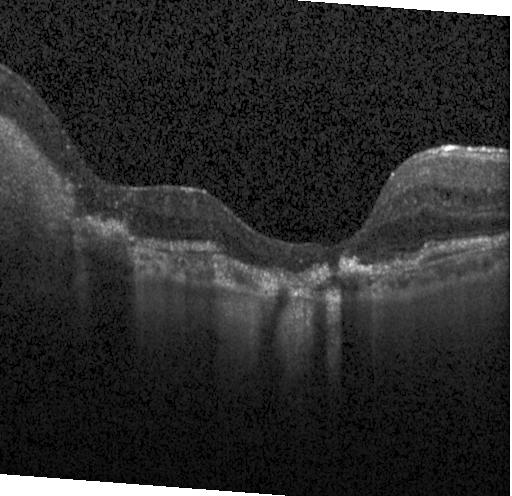 Macular OCT: a choroidal neovascular membrane.